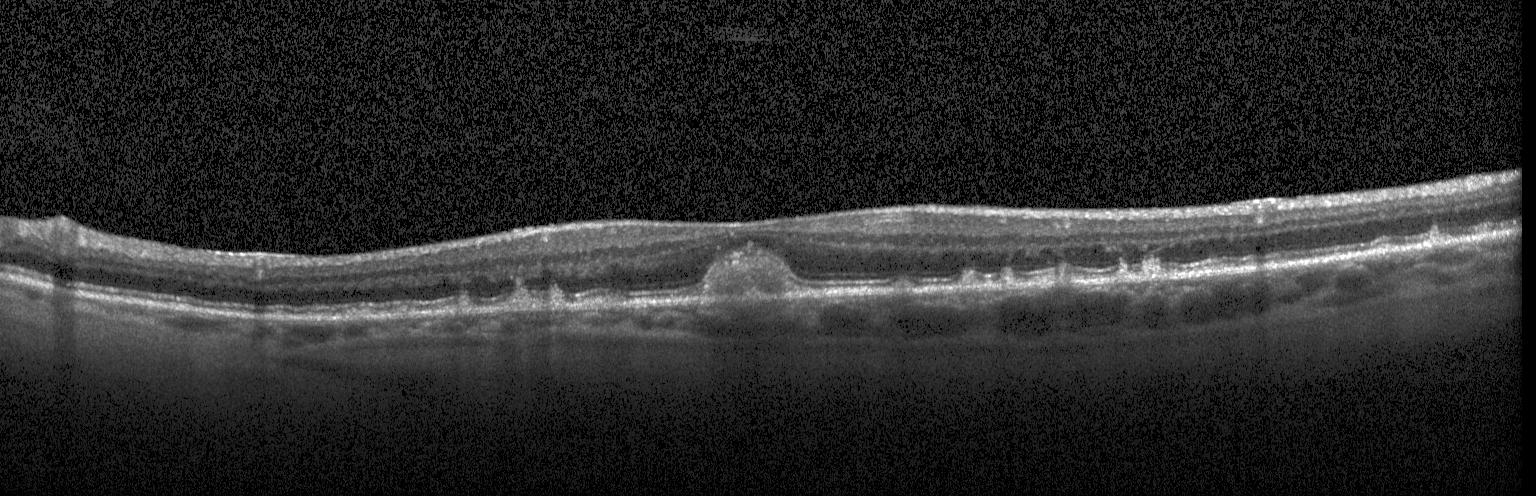
OCT scan showing a choroidal neovascular membrane.